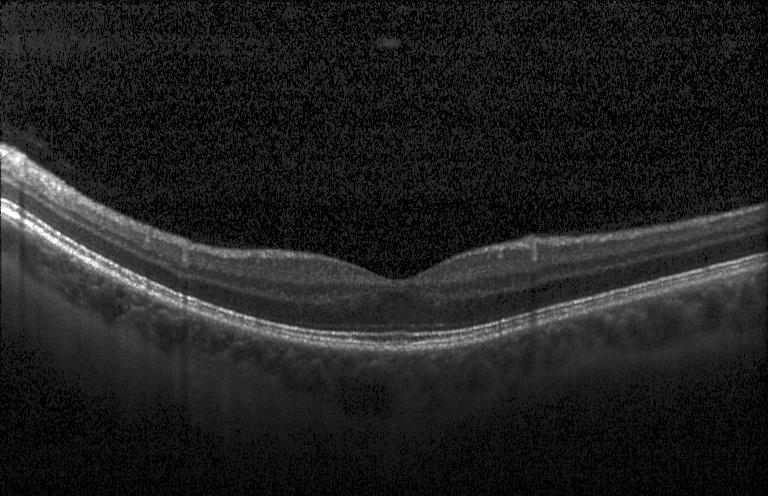
Optical coherence tomography B-scan, acquired on a Heidelberg Spectralis. Dx: no evidence of choroidal neovascularization, diabetic macular edema, or drusen.